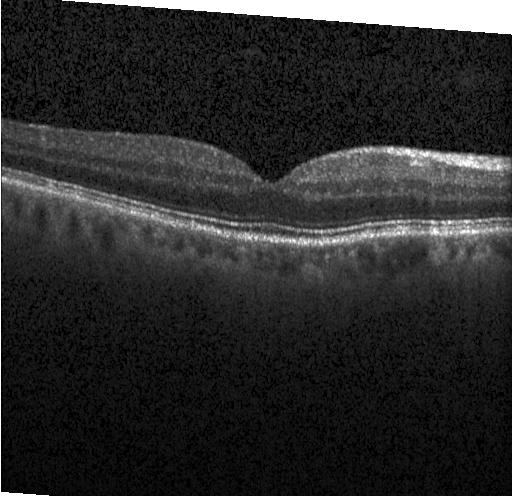

Instrument: Heidelberg Spectralis. Retinal OCT B-scan. Horizontal scan through the fovea — Impression: neither CNV, DME, nor drusen.